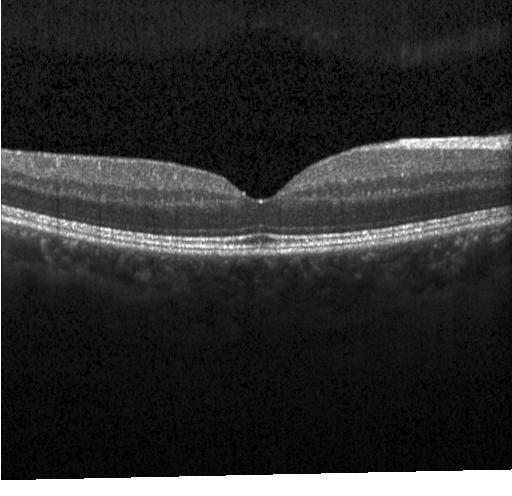
Spectral-domain OCT. Acquired on a Heidelberg Spectralis. OCT line scan. Macular scan — Impression: neither CNV, DME, nor drusen.